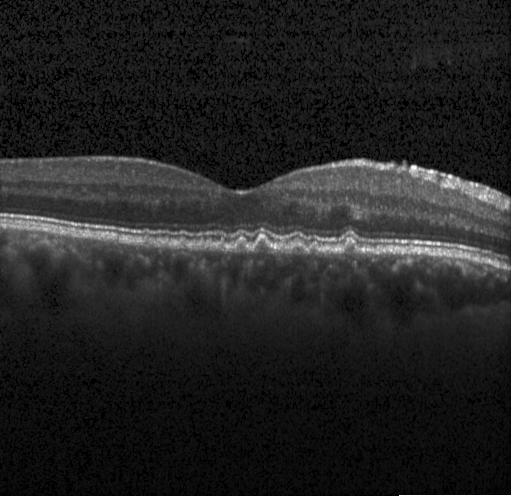
Optical coherence tomography scan
Impression: multiple drusen.